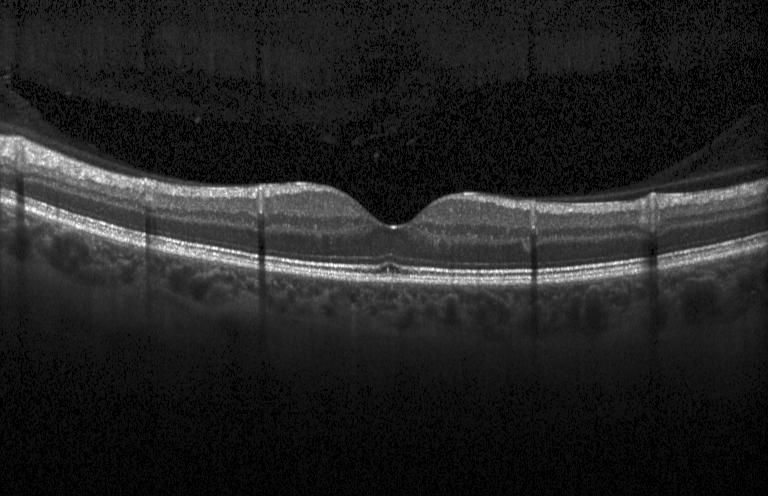
OCT B-scan showing no evidence of CNV, DME, or drusen.